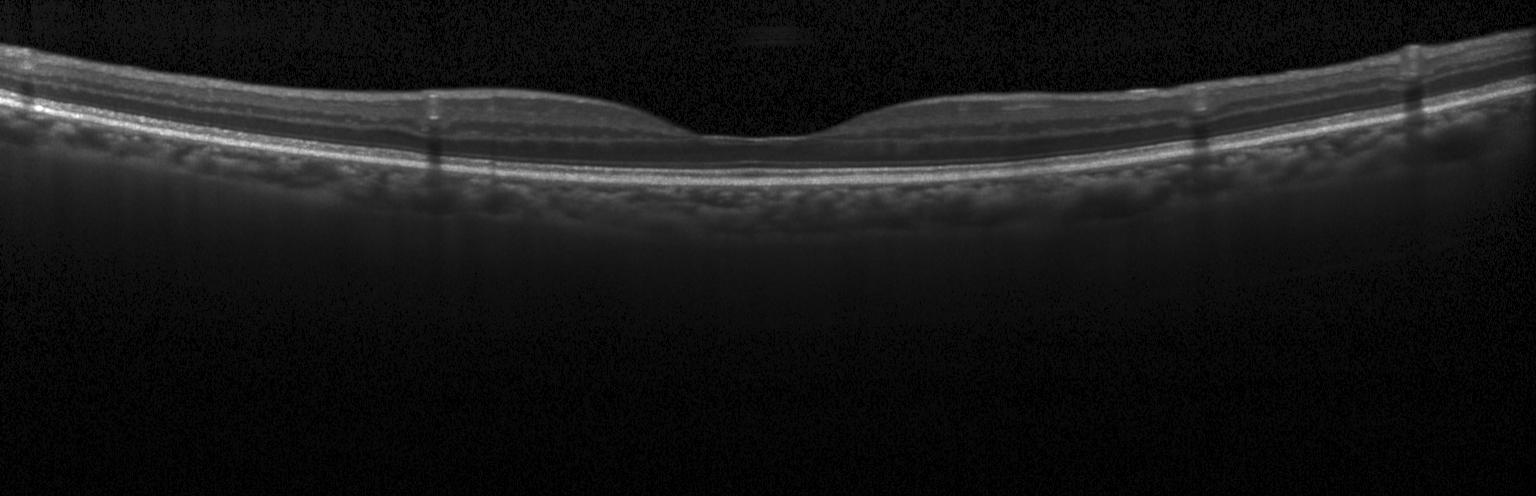 Optical coherence tomography scan; Heidelberg Spectralis.
Macular OCT: no evidence of CNV, DME, or drusen.